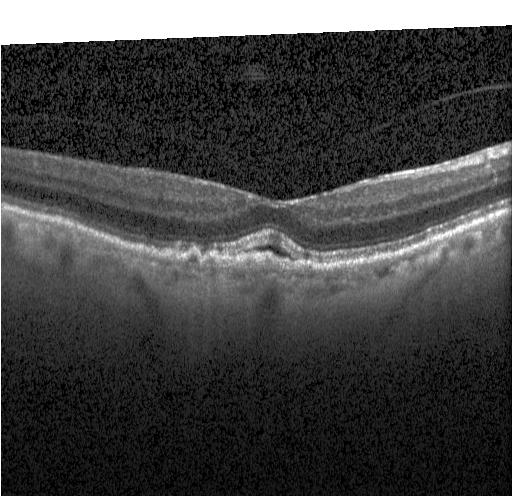 Spectral-domain optical coherence tomography; retinal OCT B-scan. Diagnosis: a choroidal neovascular membrane.